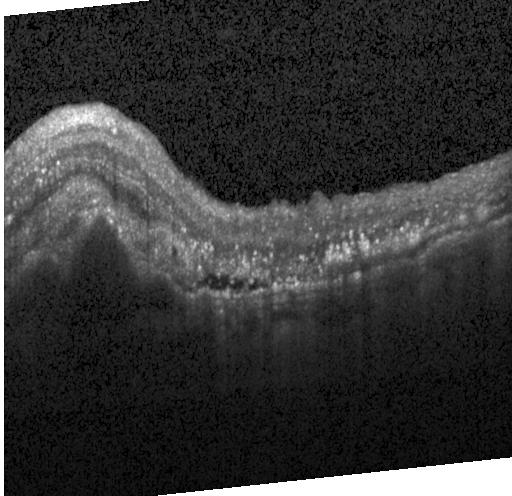 Spectral-domain optical coherence tomography; retinal OCT cross-section — Impression: choroidal neovascularization (CNV).